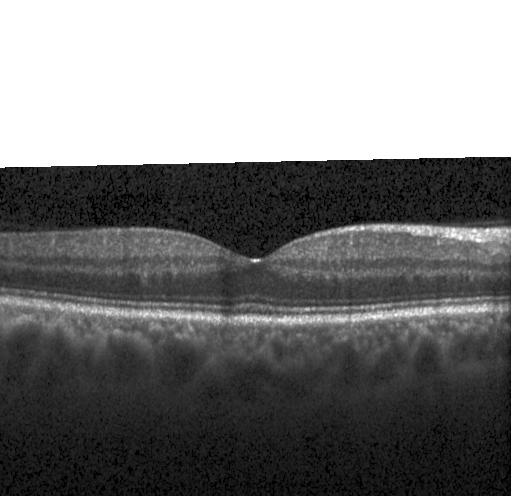
Diagnosis: no CNV, no DME, and no drusen.